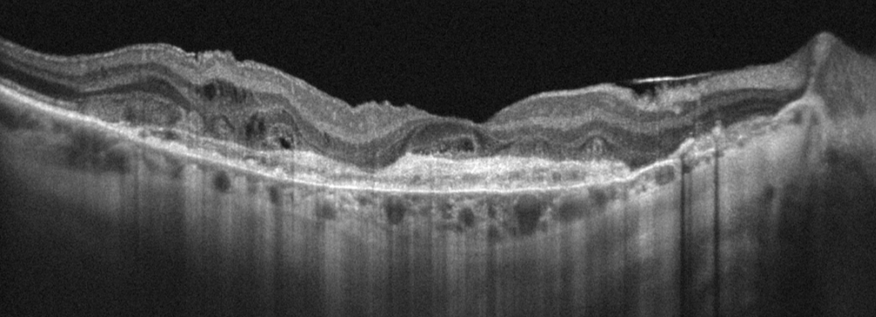 Impression: AMD.